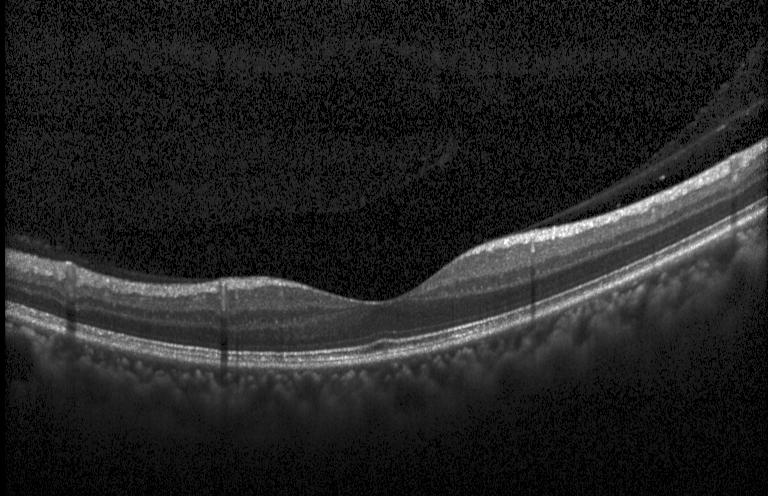

Spectral-domain optical coherence tomography · macular scan · retinal OCT cross-section.
Finding: no choroidal neovascularization, diabetic macular edema, or drusen.